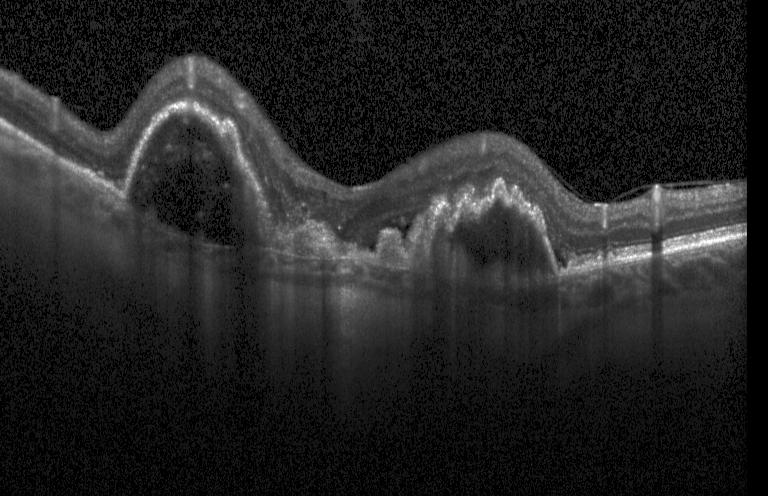

Impression: a choroidal neovascular membrane.